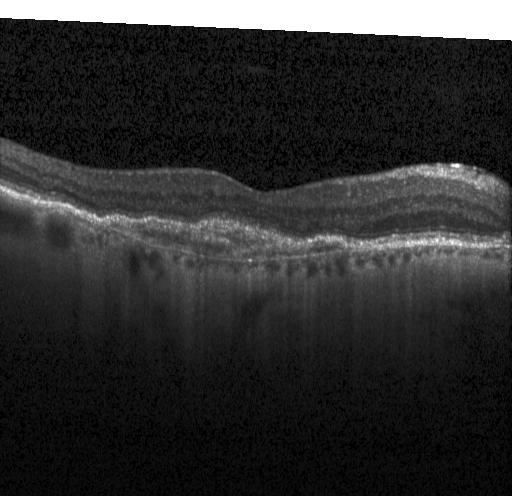

Horizontal scan through the fovea; Heidelberg Spectralis; OCT line scan.
Diagnosis: choroidal neovascularization (CNV).